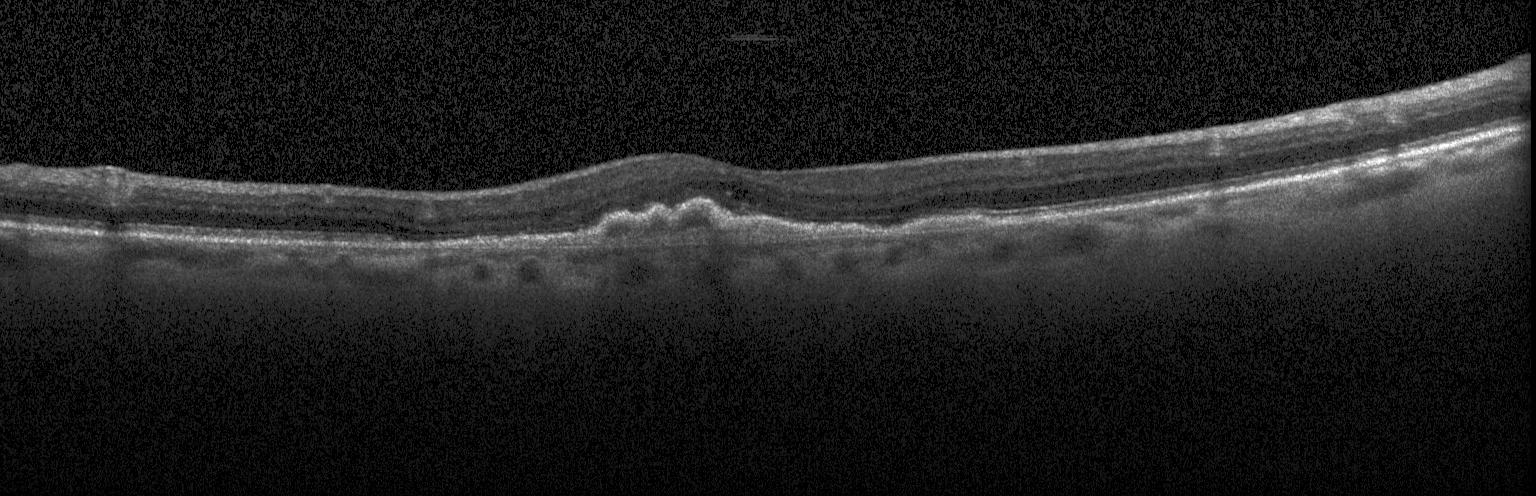
Optical coherence tomography scan. Spectral-domain optical coherence tomography.
The scan shows a choroidal neovascular membrane.